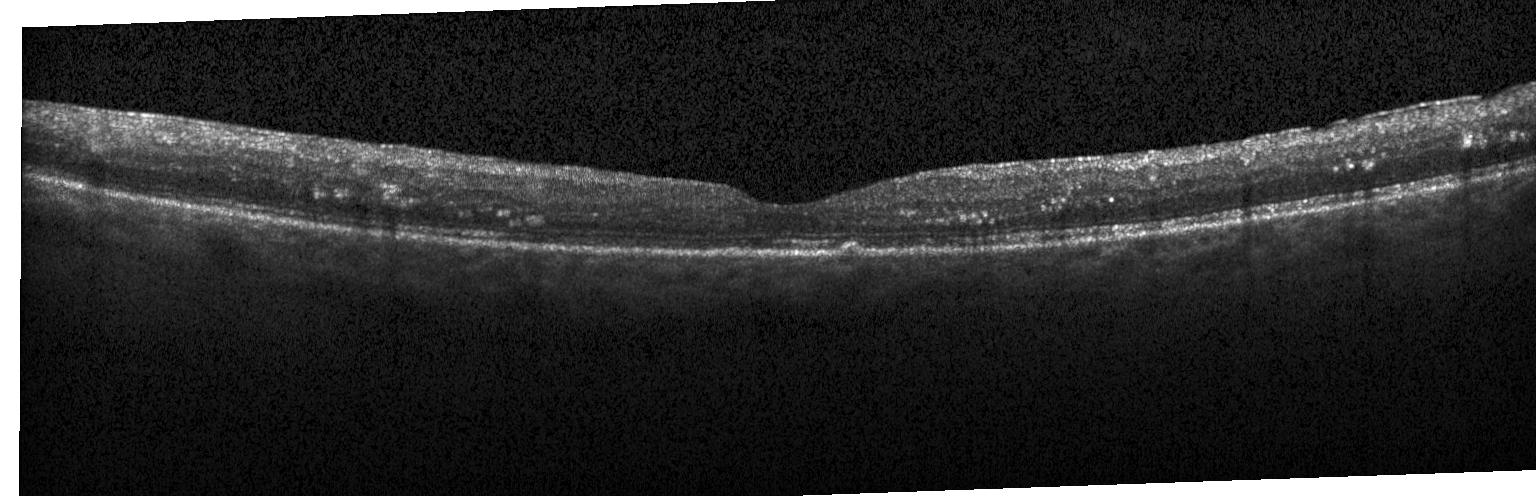
Heidelberg Spectralis · OCT B-scan — Assessment: diabetic macular edema (DME).